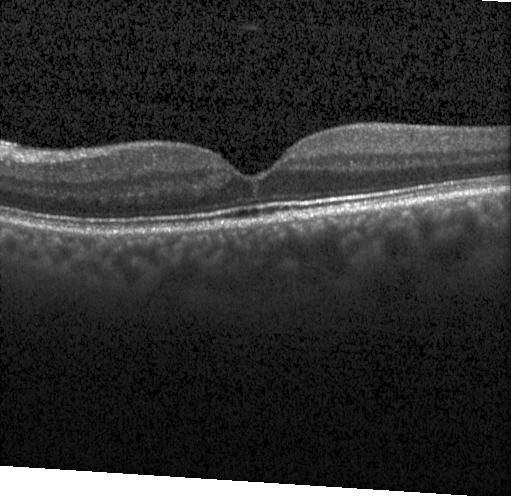
Retinal OCT cross-section. Acquired on a Heidelberg Spectralis. Diagnosis: no CNV, DME, or drusen.